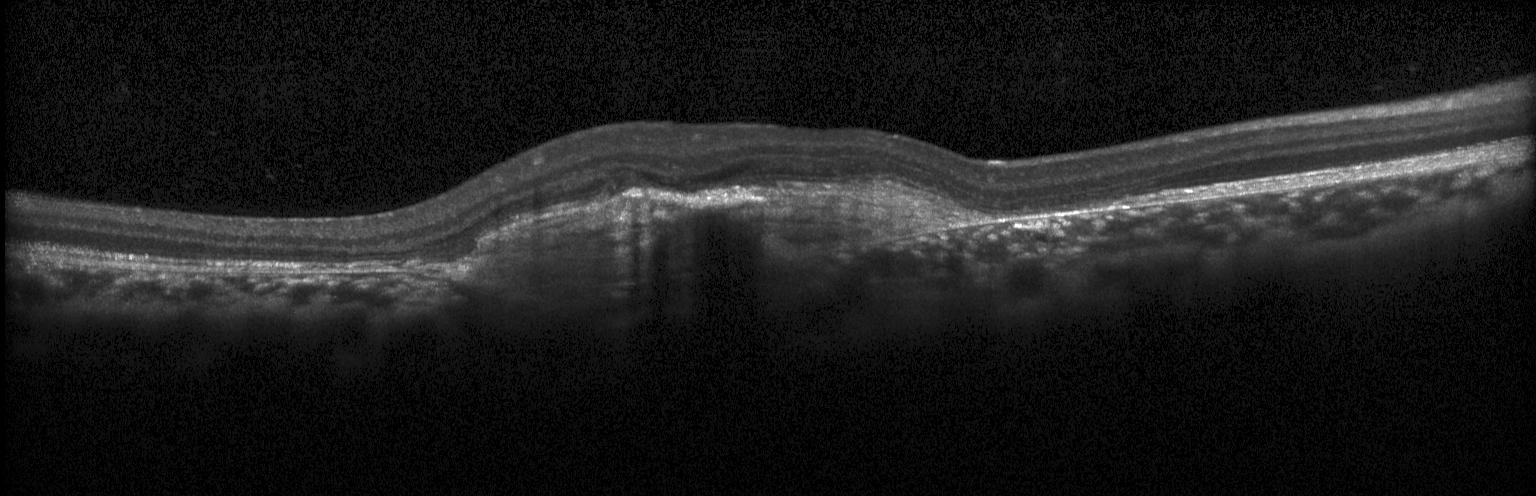 Assessment: choroidal neovascularization.